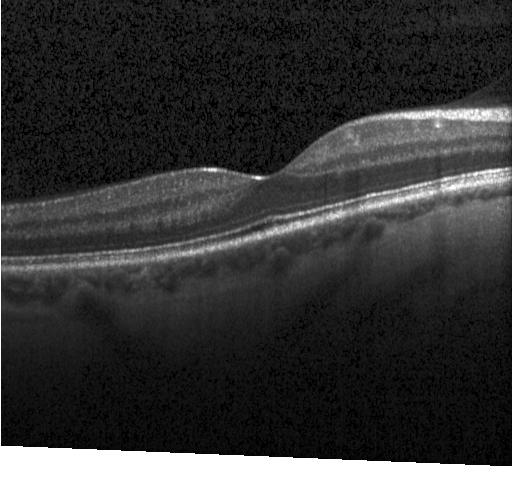

OCT B-scan · Heidelberg Spectralis · SD-OCT · fovea-centered.
Assessment: no CNV, no DME, and no drusen.